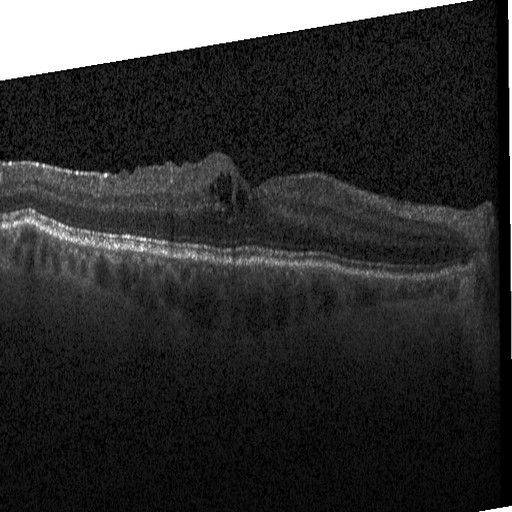
Impression: diabetic macular edema.